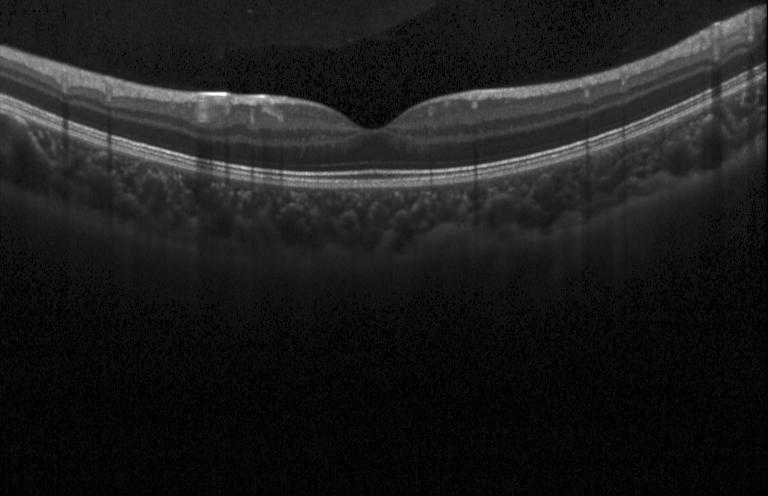

SD-OCT, optical coherence tomography scan, Heidelberg Spectralis OCT system. This B-scan demonstrates neither choroidal neovascularization, diabetic macular edema, nor drusen.